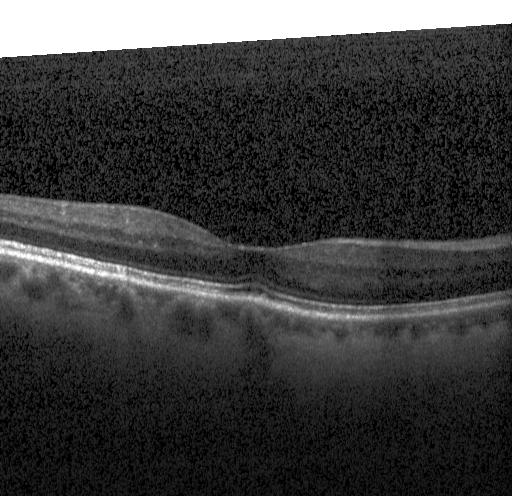

Retinal OCT cross-section, SD-OCT. Diagnosis: neither choroidal neovascularization, diabetic macular edema, nor drusen.